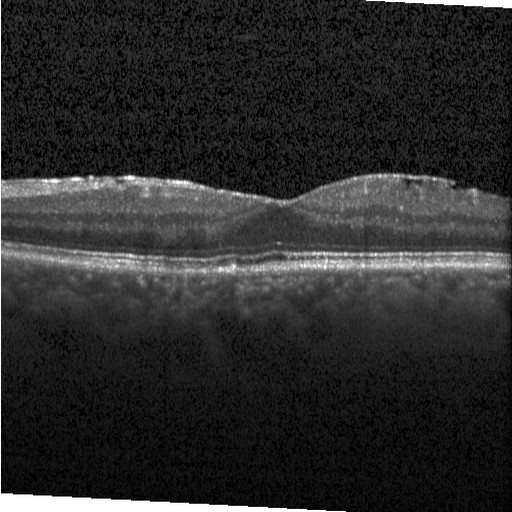

Macular OCT: DME.